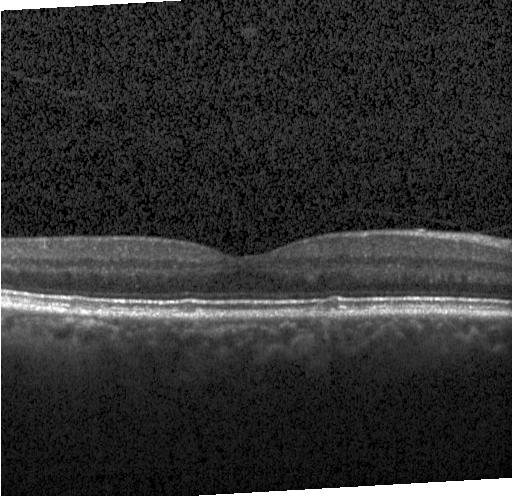 SD-OCT; acquired on a Heidelberg Spectralis; retinal OCT B-scan. OCT finding: no evidence of CNV, DME, or drusen.